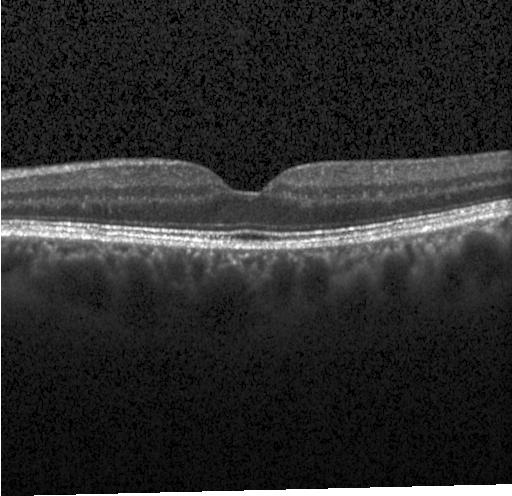
OCT finding: no evidence of CNV, DME, or drusen.